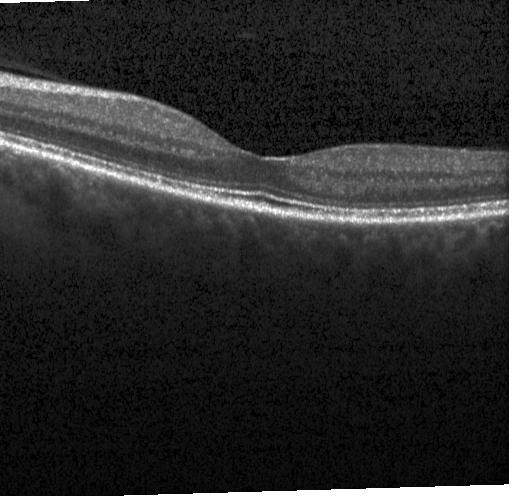

Macular scan · retinal OCT B-scan · spectral-domain OCT · acquired on a Heidelberg Spectralis — Impression: no choroidal neovascularization, no diabetic macular edema, and no drusen.